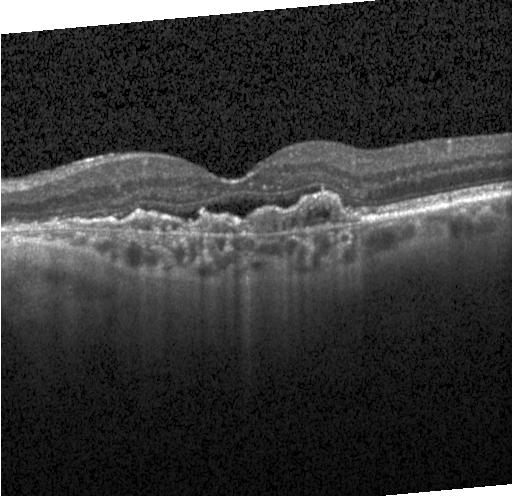
Optical coherence tomography B-scan; acquired on a Heidelberg Spectralis; spectral-domain optical coherence tomography. Assessment: a choroidal neovascular membrane.